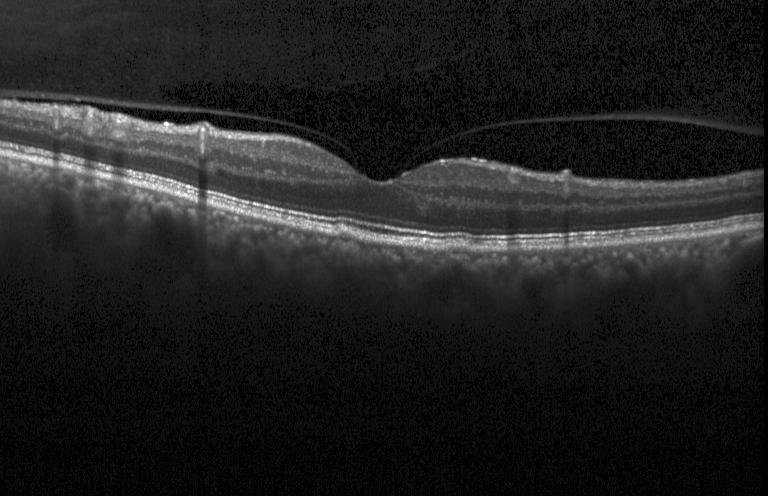
Spectral-domain OCT · retinal OCT B-scan · through the macula · Heidelberg Spectralis OCT system — Dx: sub-RPE drusenoid deposits.